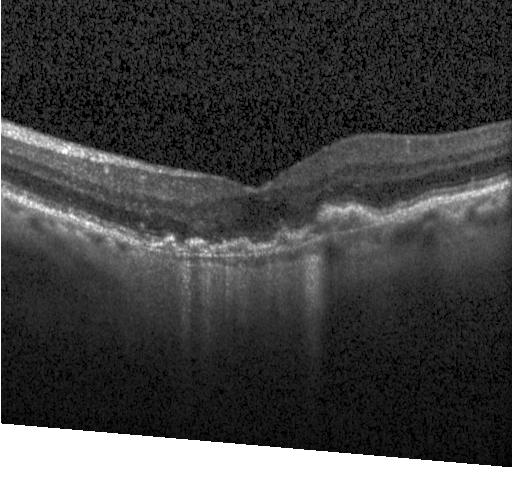

Horizontal scan through the fovea. Spectral-domain optical coherence tomography. Heidelberg Spectralis. Optical coherence tomography scan — Finding: choroidal neovascularization.